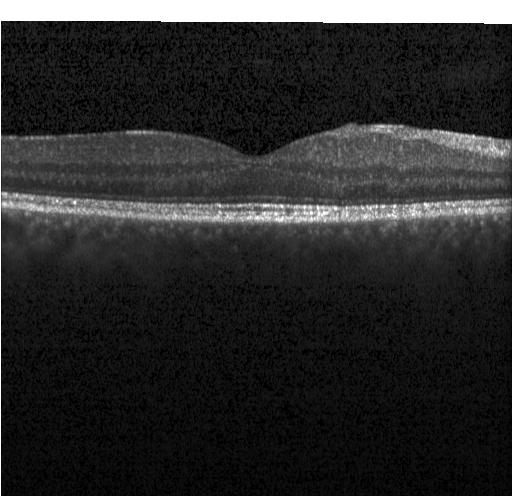

Optical coherence tomography scan. No choroidal neovascularization, no diabetic macular edema, and no drusen.